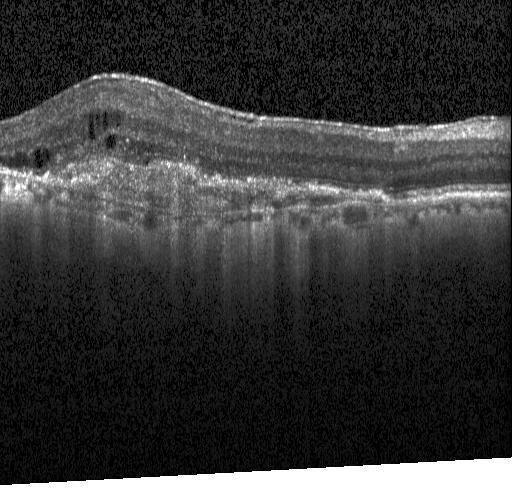

Finding: a choroidal neovascular membrane.